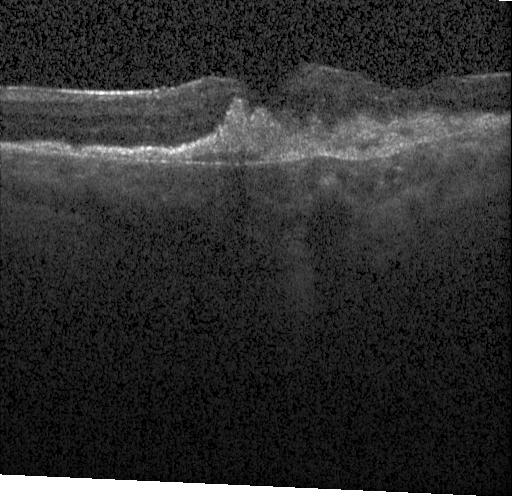

Through the macula; optical coherence tomography scan — Choroidal neovascularization (CNV).